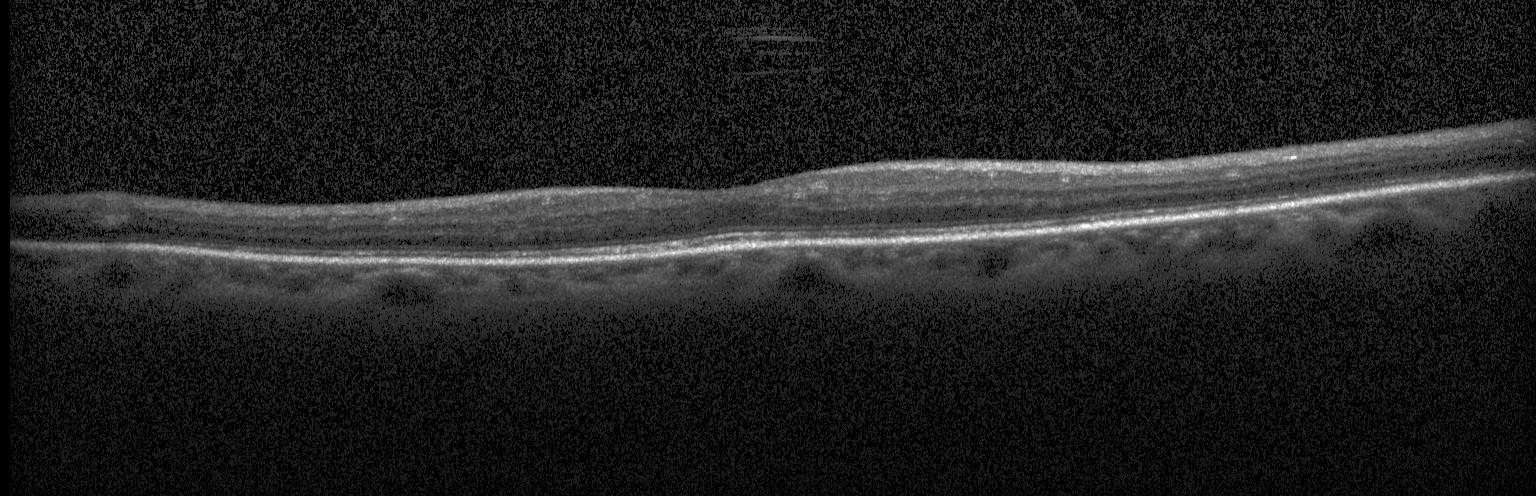 Diagnosis: neither choroidal neovascularization, diabetic macular edema, nor drusen.